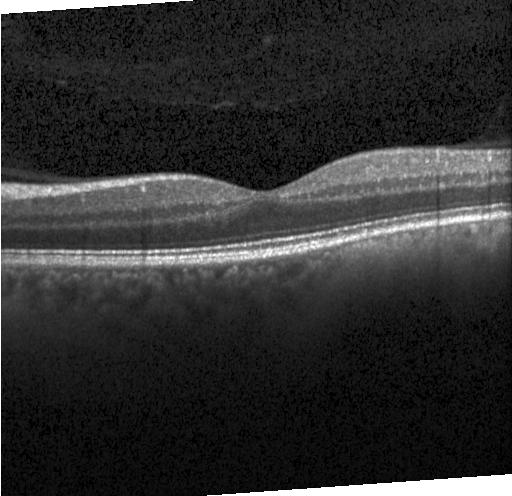

No choroidal neovascularization, no diabetic macular edema, and no drusen.